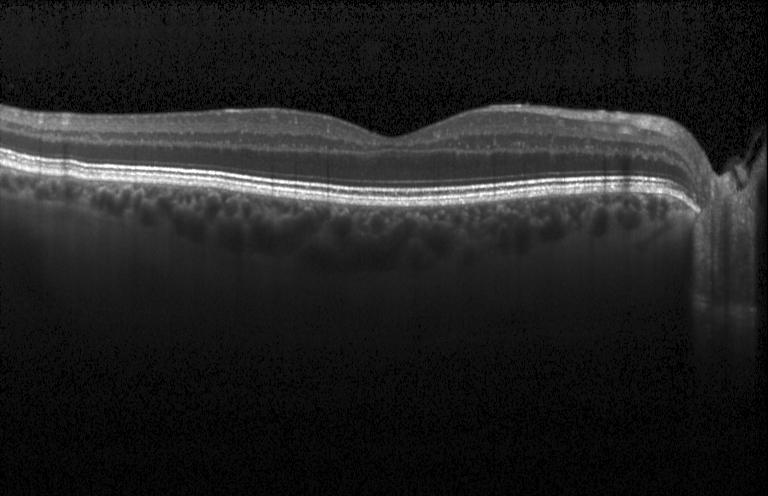

Assessment: no choroidal neovascularization, no diabetic macular edema, and no drusen.